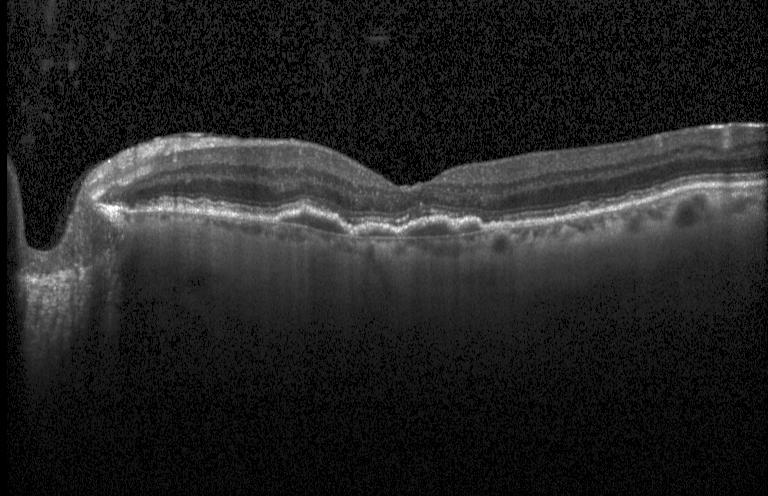

Retinal OCT cross-section, acquired on a Heidelberg Spectralis, horizontal scan through the fovea
This B-scan demonstrates CNV.